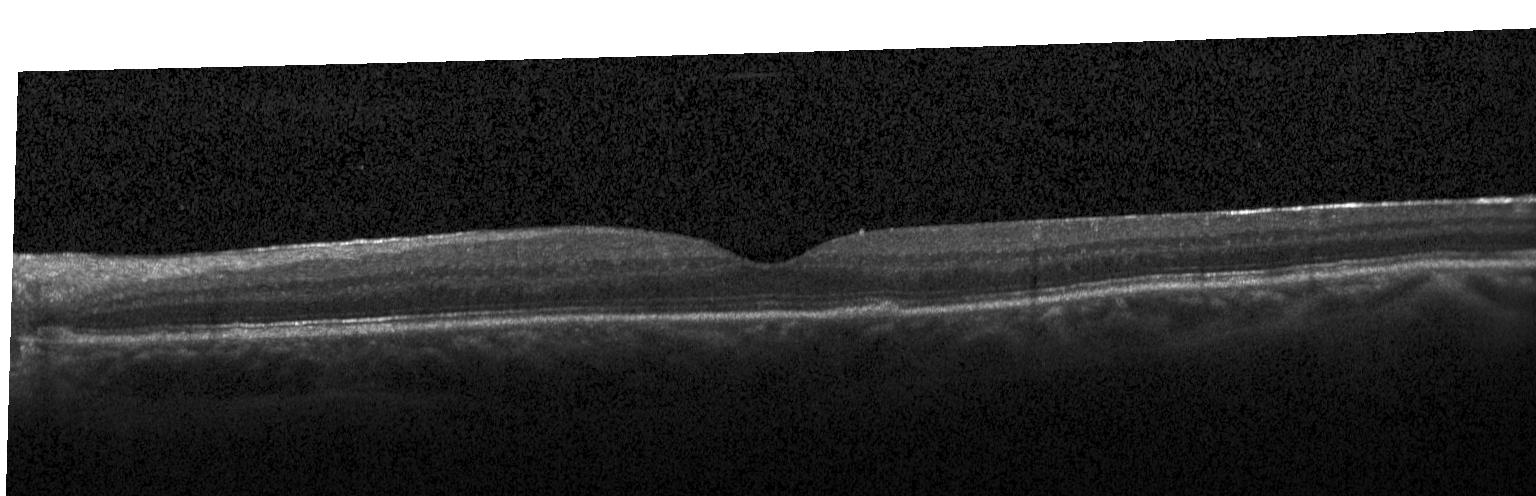
Optical coherence tomography scan · fovea-centered — Impression: multiple drusen.